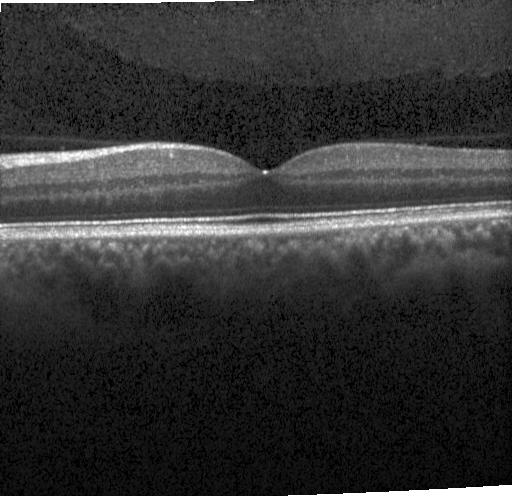
OCT line scan, macular scan, instrument: Heidelberg Spectralis. Diagnosis: no evidence of choroidal neovascularization, diabetic macular edema, or drusen.